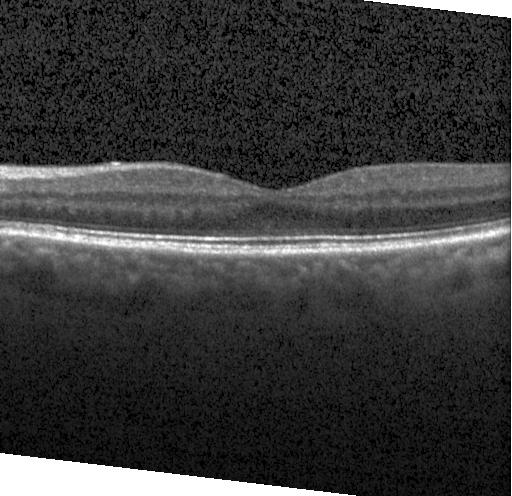

Heidelberg Spectralis; spectral-domain OCT; retinal OCT cross-section.
Diagnosis: no choroidal neovascularization, no diabetic macular edema, and no drusen.